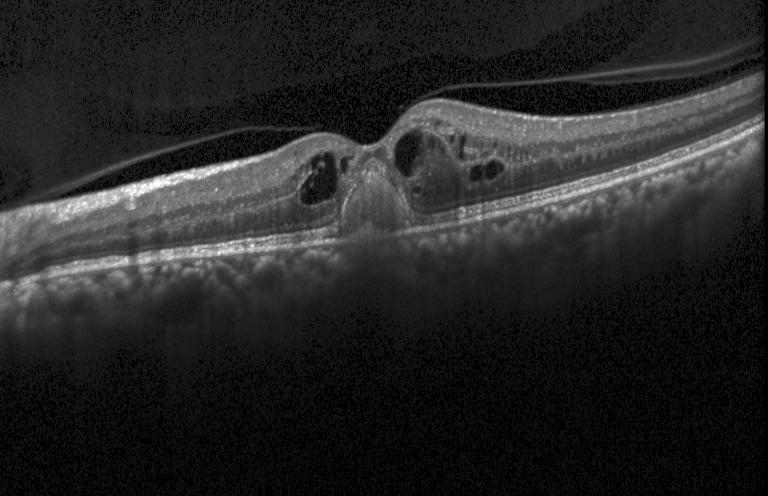

Spectral-domain optical coherence tomography · retinal OCT B-scan · acquired on a Heidelberg Spectralis · centered on the fovea. Finding: choroidal neovascularization (CNV).